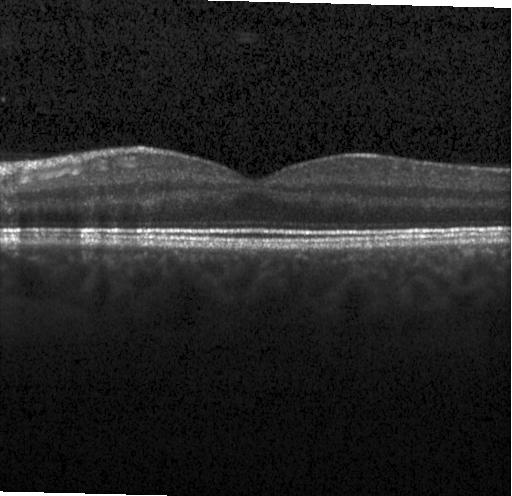

Retinal OCT B-scan.
Impression: no choroidal neovascularization, diabetic macular edema, or drusen.